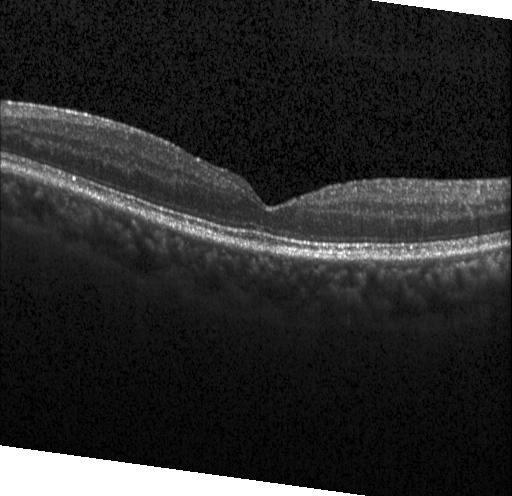

Finding: no evidence of CNV, DME, or drusen.